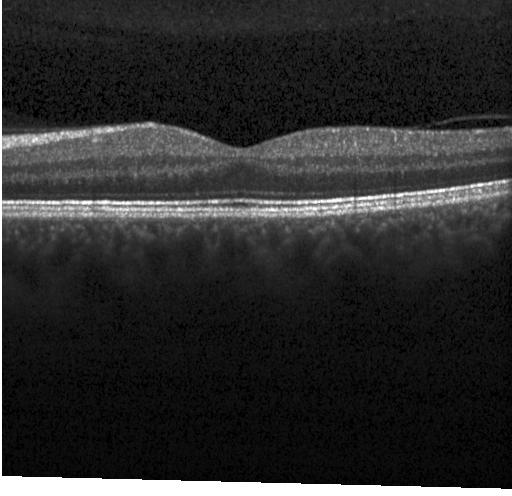
Instrument: Heidelberg Spectralis, macular scan, spectral-domain optical coherence tomography, OCT line scan. Finding: no evidence of choroidal neovascularization, diabetic macular edema, or drusen.